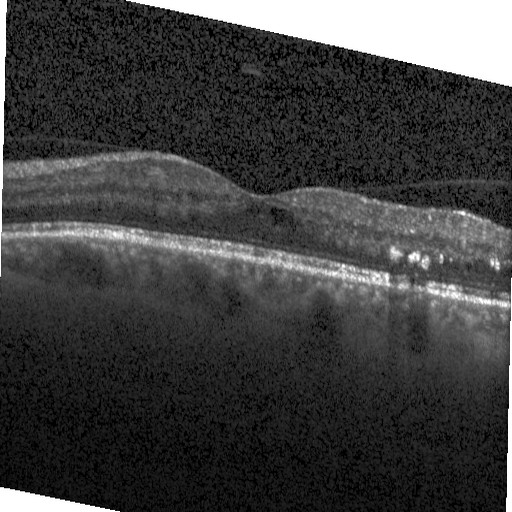

Assessment: DME.